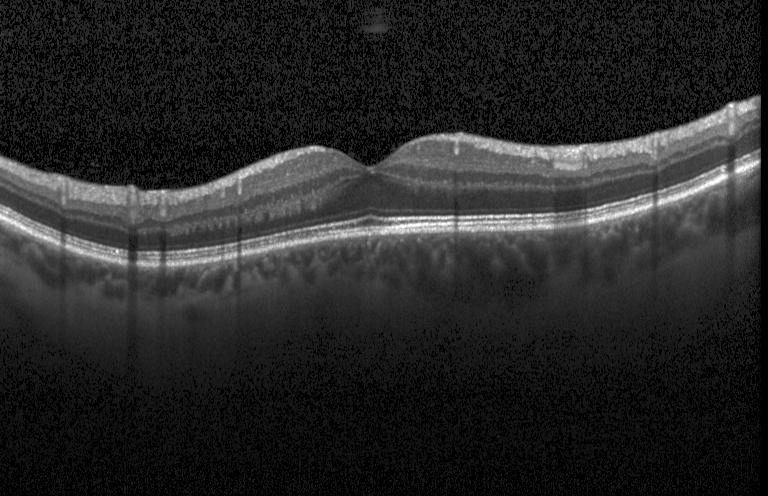 Acquired on a Heidelberg Spectralis, retinal OCT cross-section, spectral-domain optical coherence tomography, macular scan.
Diagnosis: no choroidal neovascularization, no diabetic macular edema, and no drusen.